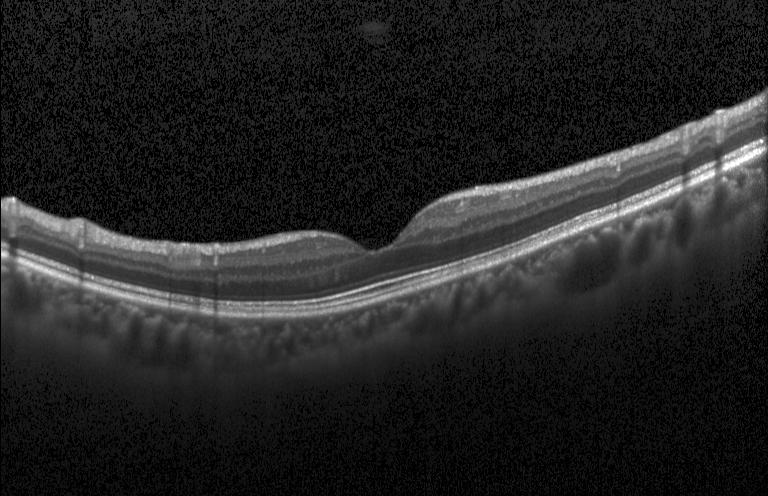

Fovea-centered, OCT B-scan. OCT finding: no CNV, DME, or drusen.